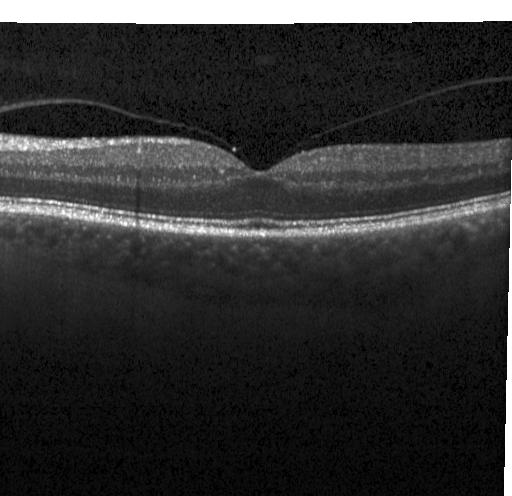 Heidelberg Spectralis; retinal OCT B-scan; centered on the fovea; SD-OCT.
This B-scan demonstrates no evidence of choroidal neovascularization, diabetic macular edema, or drusen.